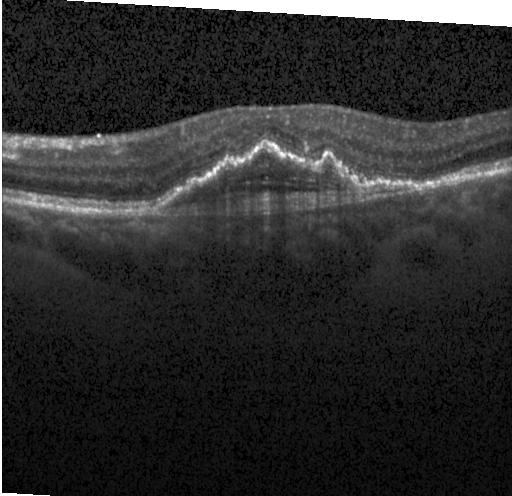

OCT B-scan. Heidelberg Spectralis OCT system. Spectral-domain optical coherence tomography. Through the macula. Assessment: a choroidal neovascular membrane.